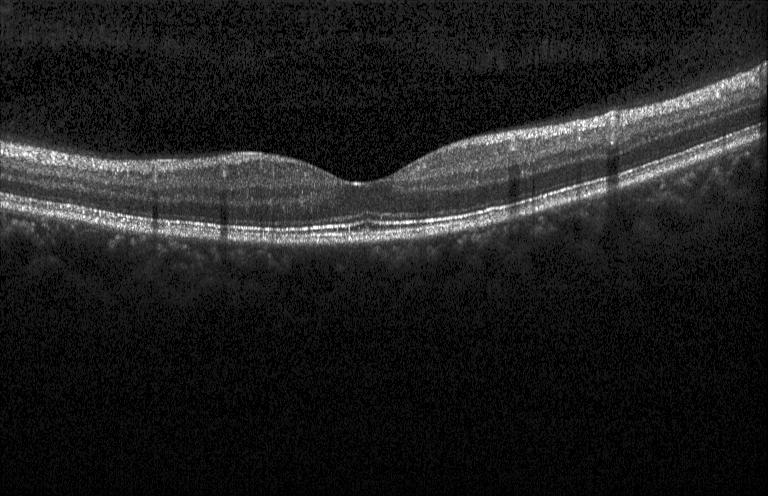
Diagnosis: no choroidal neovascularization, no diabetic macular edema, and no drusen.